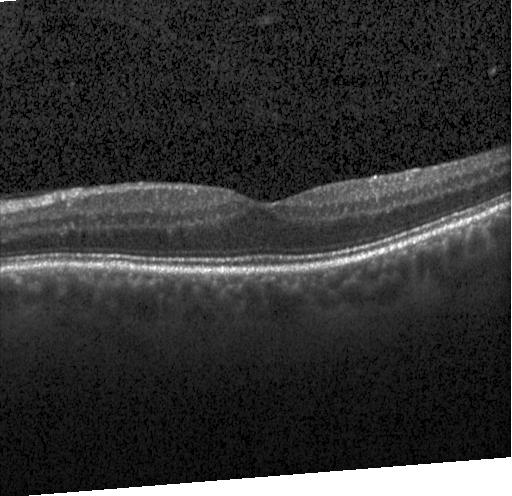 OCT B-scan.
The scan shows no choroidal neovascularization, diabetic macular edema, or drusen.